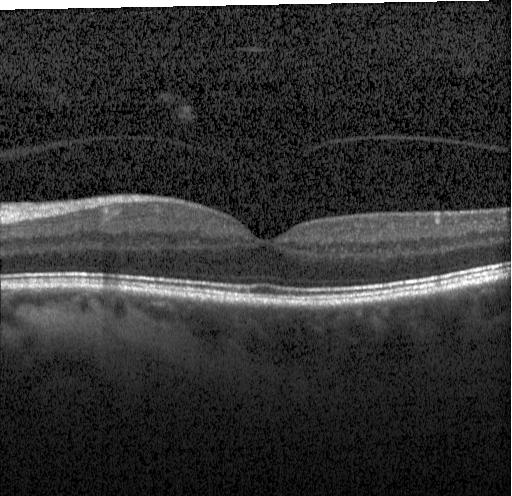
OCT B-scan; SD-OCT; instrument: Heidelberg Spectralis.
Diagnosis: neither choroidal neovascularization, diabetic macular edema, nor drusen.